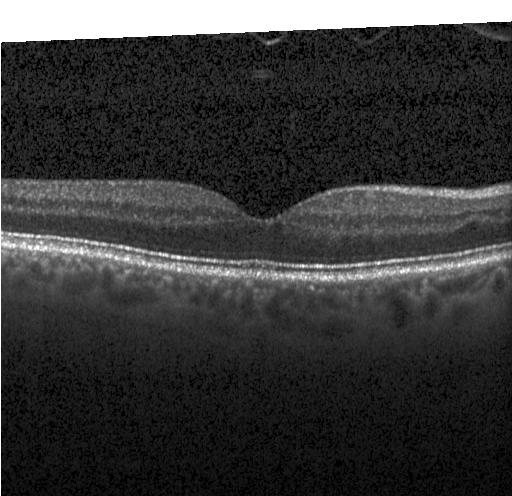

OCT line scan · instrument: Heidelberg Spectralis. The scan shows no choroidal neovascularization, no diabetic macular edema, and no drusen.